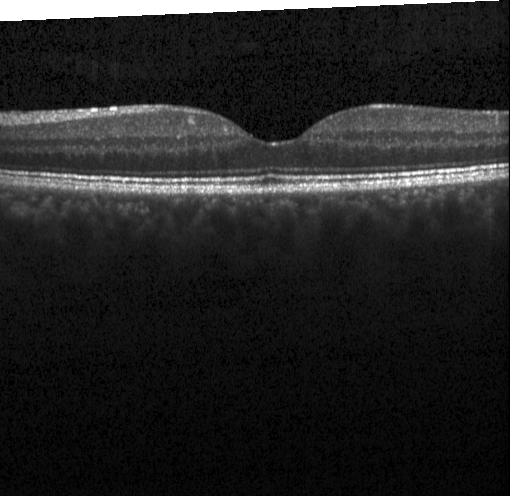 Centered on the fovea. Optical coherence tomography scan
Macular OCT: no evidence of choroidal neovascularization, diabetic macular edema, or drusen.